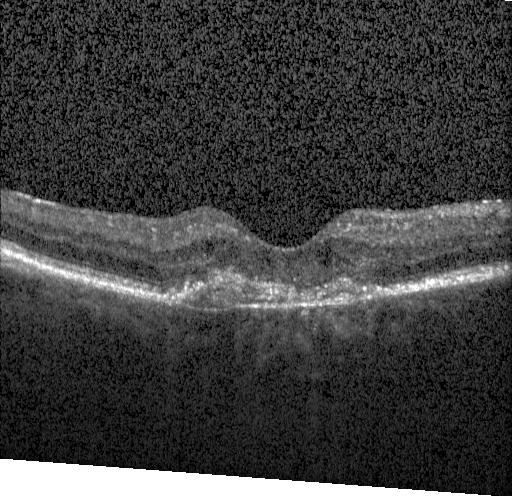

Retinal OCT cross-section showing CNV.